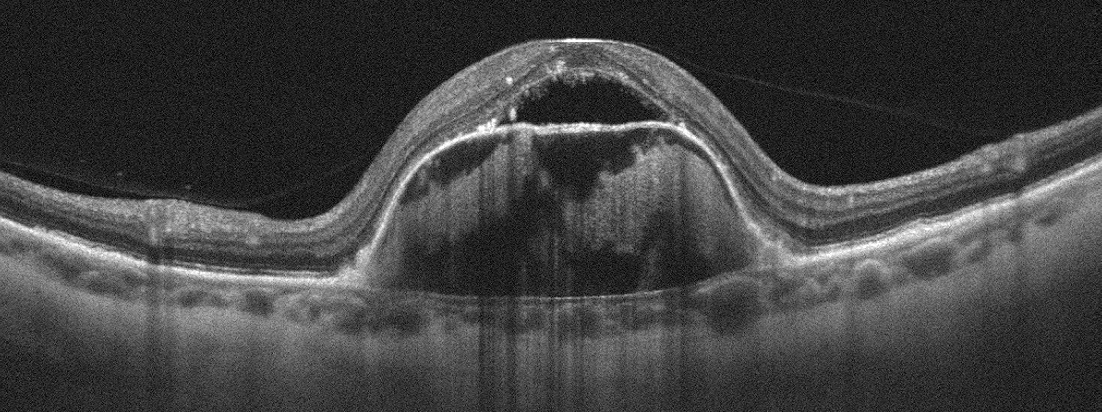

Fovea-centered, Optovue Avanti RTVue XR, OCT B-scan.
OCT finding: AMD.